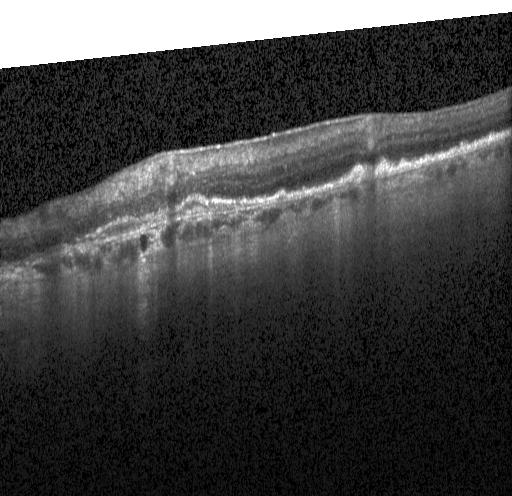
OCT B-scan.
Impression: choroidal neovascularization (CNV).